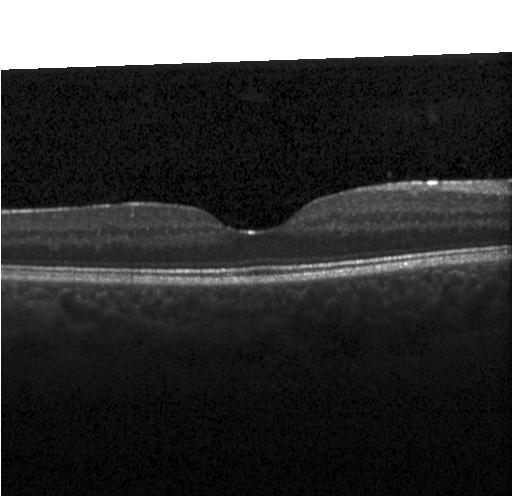

OCT scan showing no evidence of choroidal neovascularization, diabetic macular edema, or drusen.